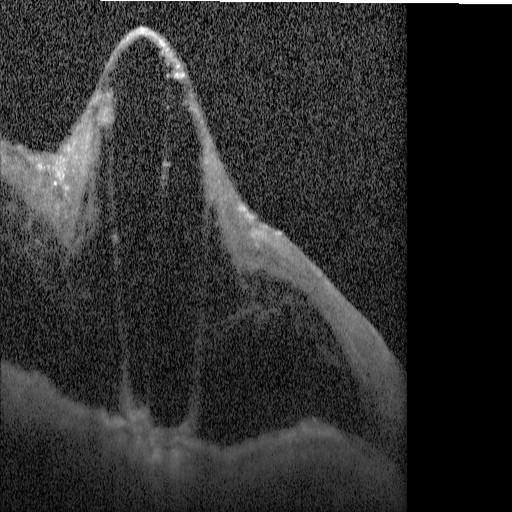
DME.